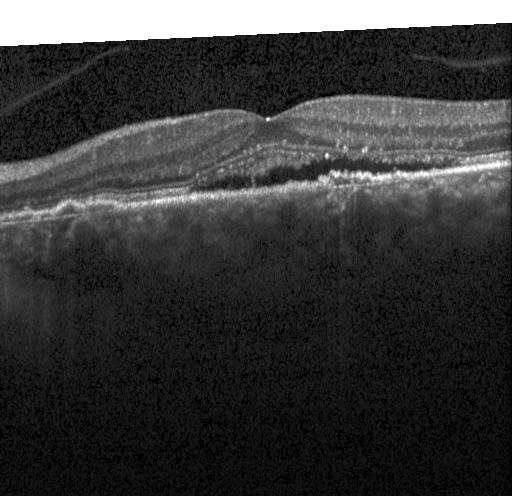

Instrument: Heidelberg Spectralis, spectral-domain OCT, horizontal scan through the fovea, OCT B-scan. A choroidal neovascular membrane.